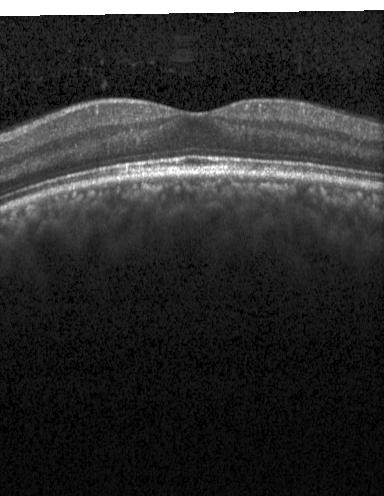

Retinal OCT cross-section.
Assessment: no choroidal neovascularization, no diabetic macular edema, and no drusen.